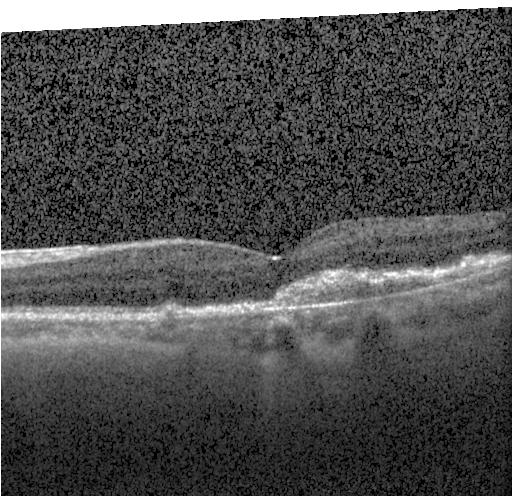 Retinal OCT B-scan · through the macula · acquired on a Heidelberg Spectralis. Impression: a choroidal neovascular membrane.